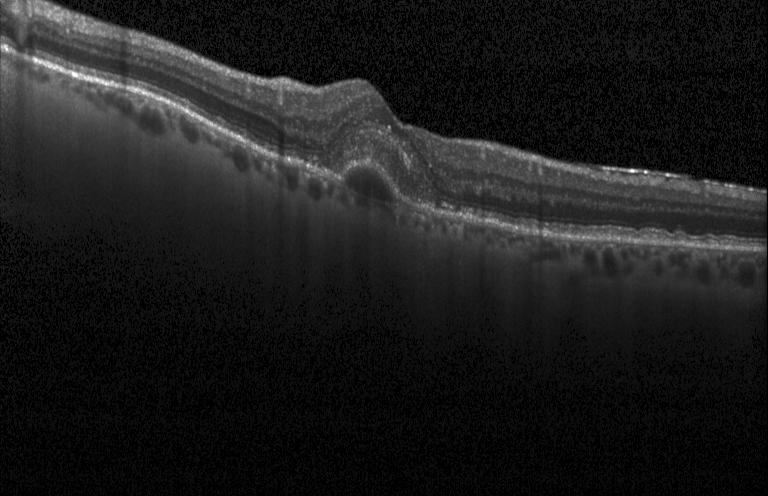
Assessment: a choroidal neovascular membrane.